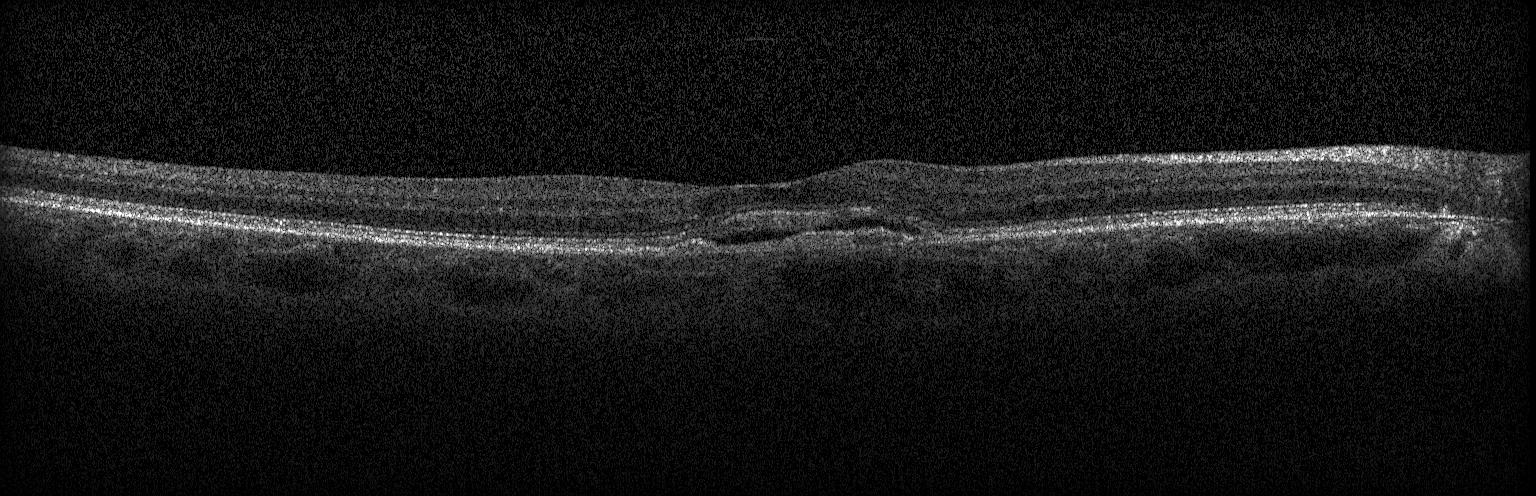 Heidelberg Spectralis. Optical coherence tomography scan
This B-scan demonstrates a choroidal neovascular membrane.